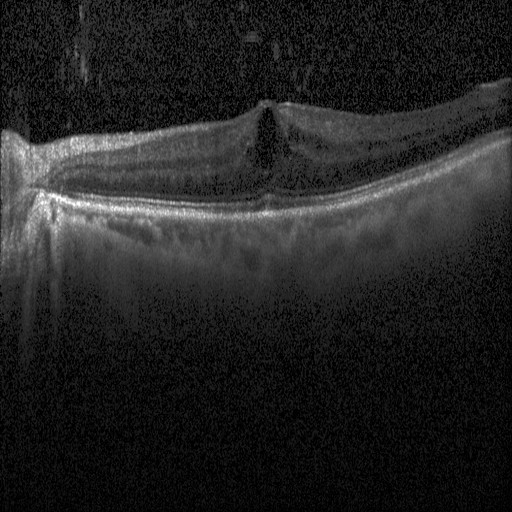

Dx: diabetic macular edema (DME).